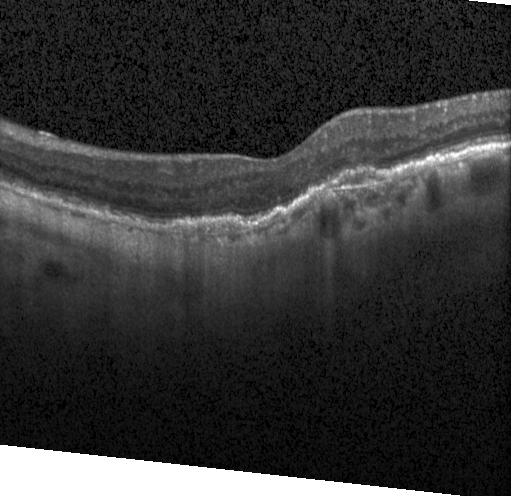

Spectral-domain OCT · optical coherence tomography scan · centered on the fovea
Dx: choroidal neovascularization.